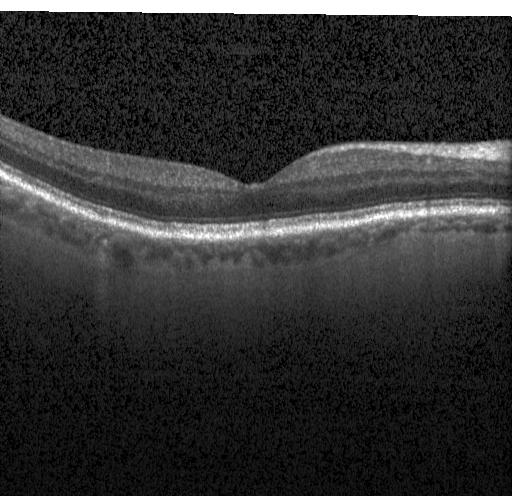
Spectral-domain optical coherence tomography, retinal OCT cross-section. Macular OCT: no choroidal neovascularization, no diabetic macular edema, and no drusen.